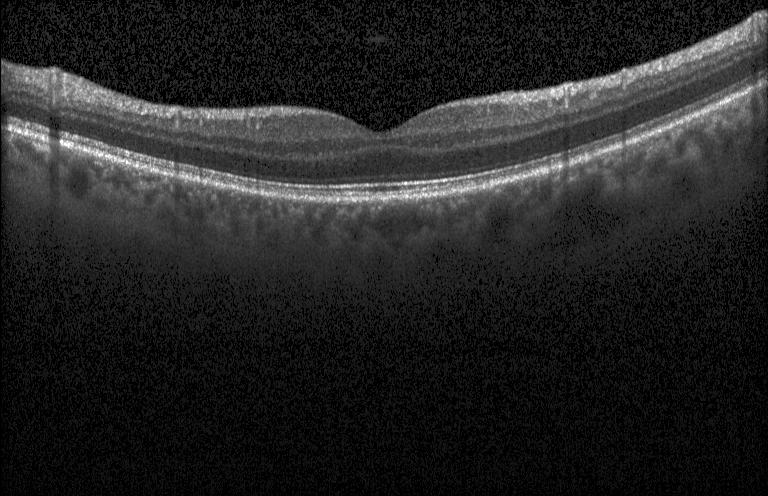 The scan shows no evidence of CNV, DME, or drusen.